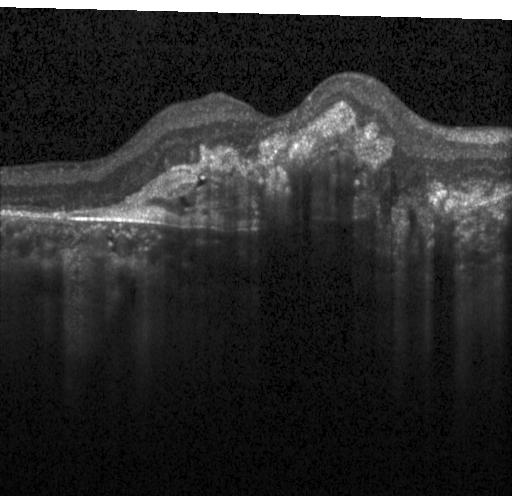

Optical coherence tomography B-scan. Impression: a choroidal neovascular membrane.